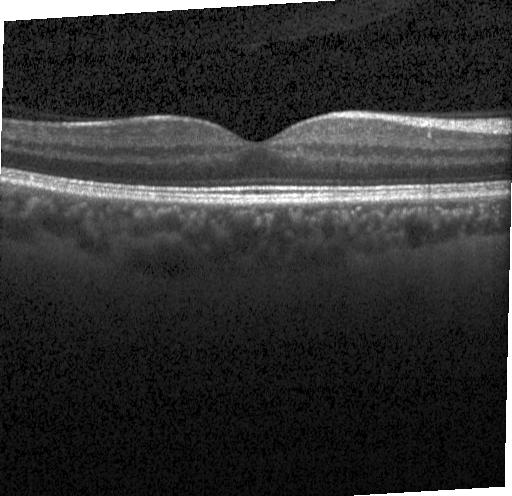
Macular OCT: neither choroidal neovascularization, diabetic macular edema, nor drusen.